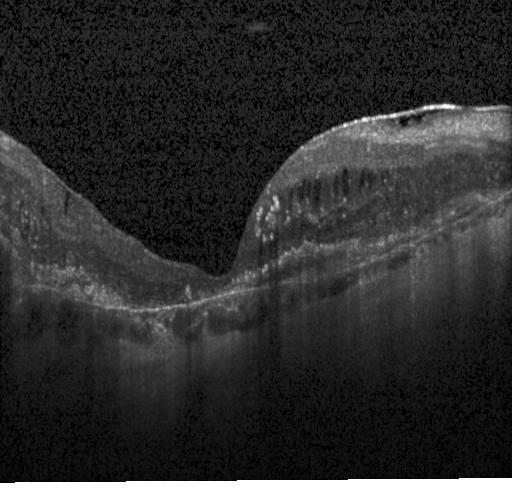
Assessment: a choroidal neovascular membrane.